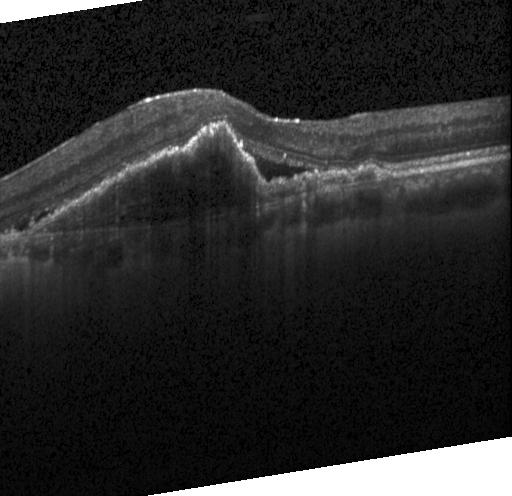
OCT B-scan
Assessment: CNV.